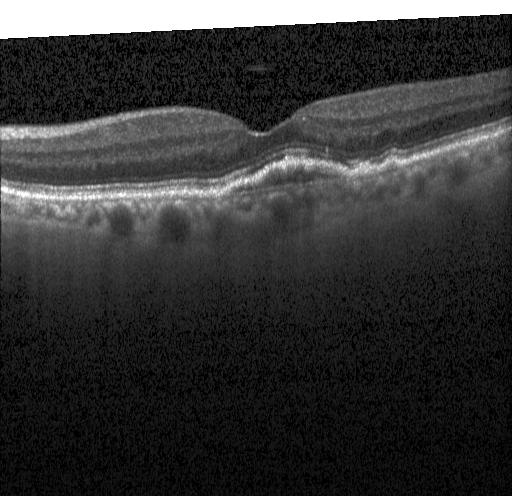
Macular scan · retinal OCT B-scan · acquired on a Heidelberg Spectralis · SD-OCT — OCT finding: a choroidal neovascular membrane.